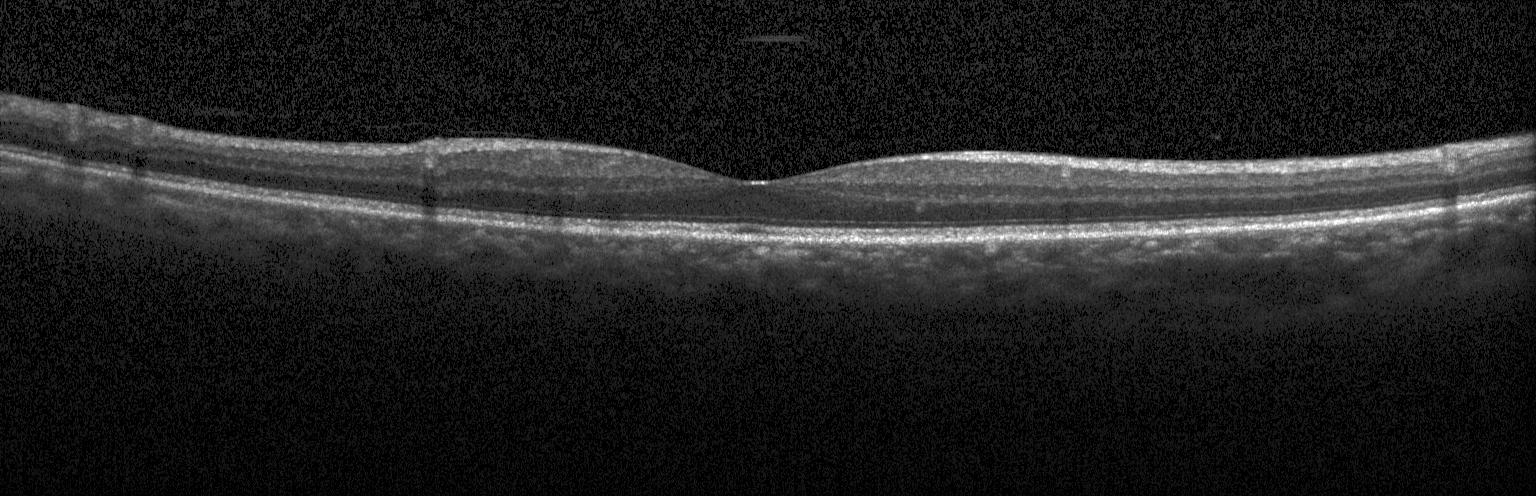

Dx: neither choroidal neovascularization, diabetic macular edema, nor drusen.